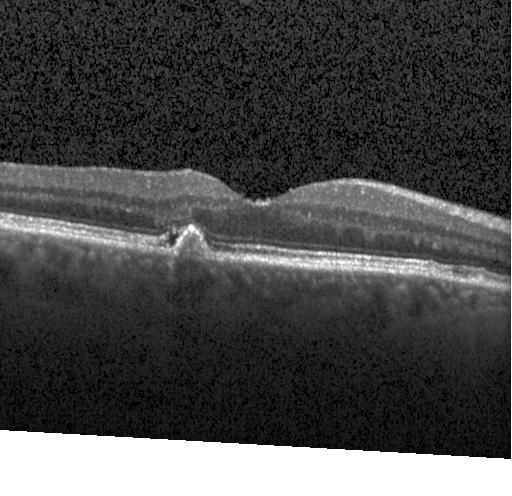 Macular scan. Acquired on a Heidelberg Spectralis. OCT line scan
Dx: a choroidal neovascular membrane.